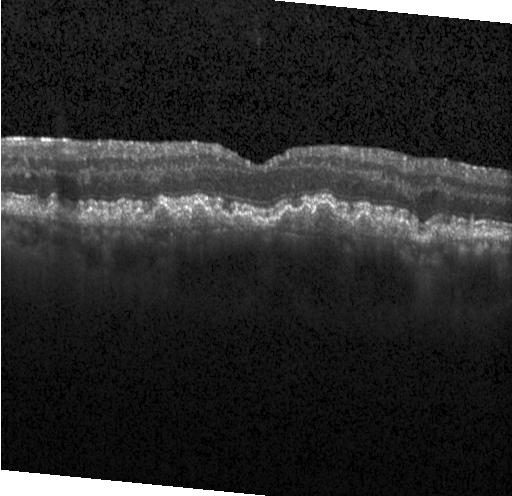
Centered on the fovea; spectral-domain optical coherence tomography; instrument: Heidelberg Spectralis; retinal OCT B-scan
Finding: CNV.